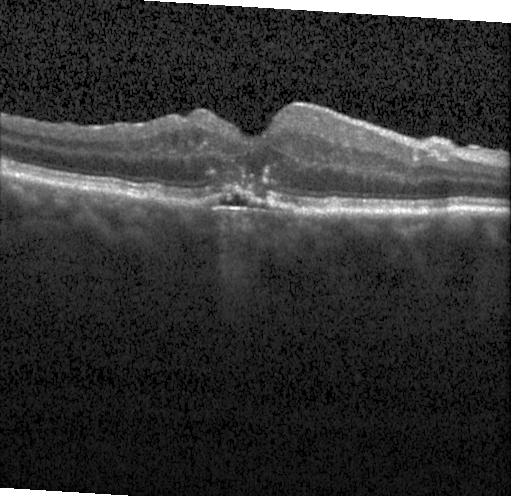

Optical coherence tomography B-scan. SD-OCT. Heidelberg Spectralis OCT system.
This B-scan demonstrates a choroidal neovascular membrane.